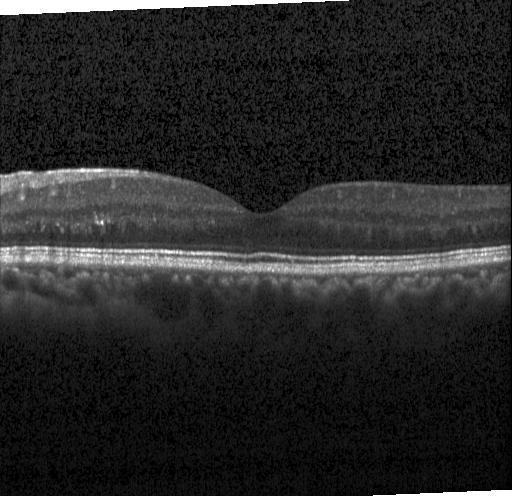 Spectral-domain OCT. OCT line scan. Fovea-centered
Impression: no evidence of choroidal neovascularization, diabetic macular edema, or drusen.